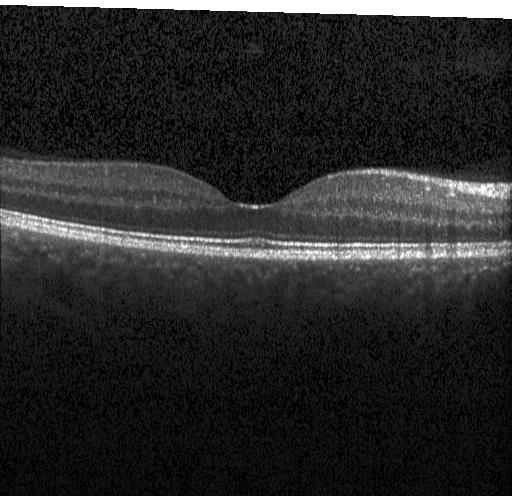

Macular OCT demonstrating no CNV, no DME, and no drusen.